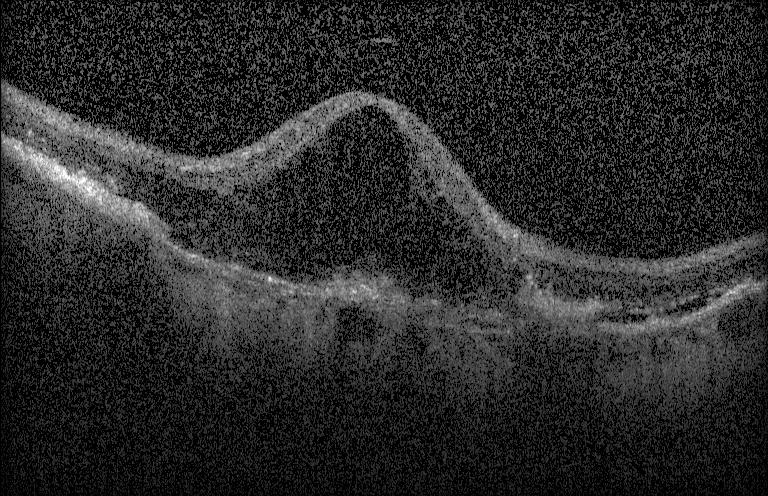
This B-scan demonstrates choroidal neovascularization (CNV).